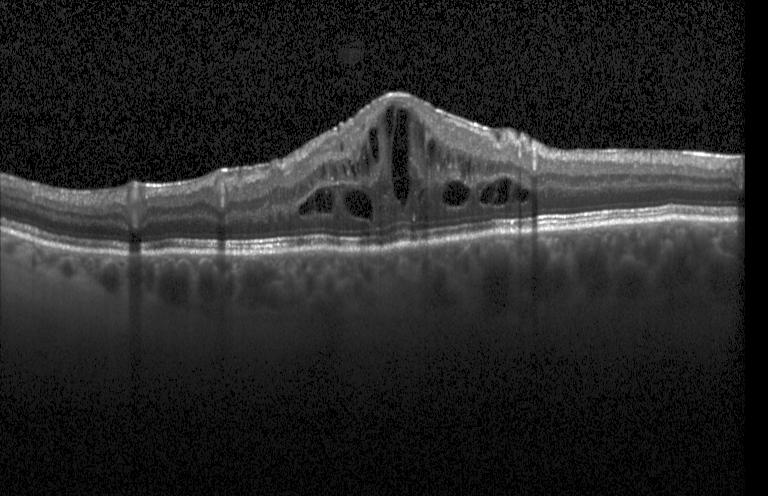 Retinal OCT cross-section · through the macula.
This B-scan demonstrates diabetic macular edema.